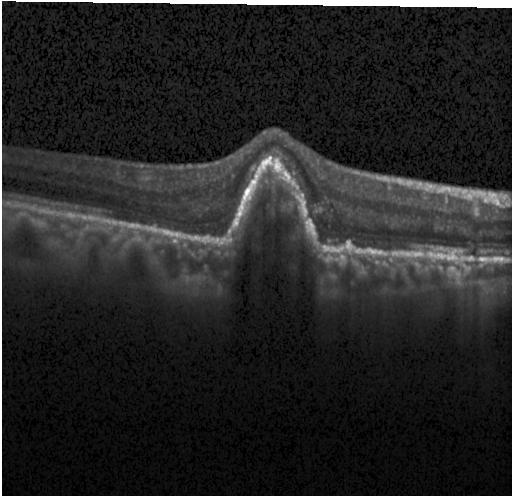

Finding: choroidal neovascularization (CNV).